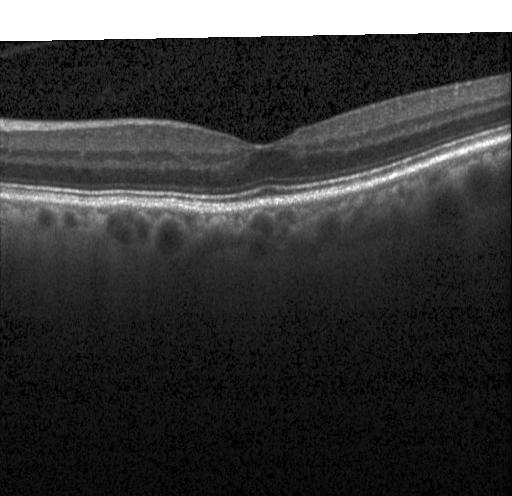

OCT scan showing no choroidal neovascularization, diabetic macular edema, or drusen.